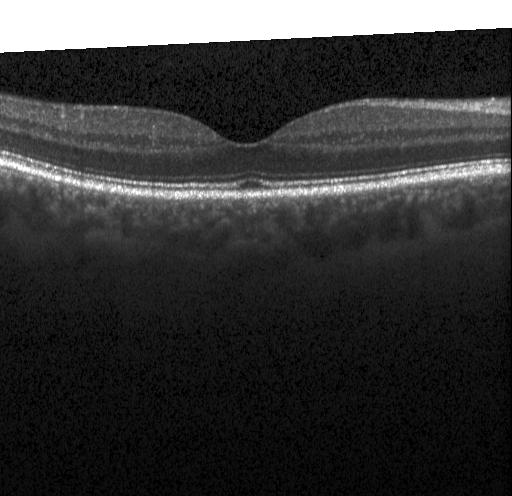

The scan shows neither choroidal neovascularization, diabetic macular edema, nor drusen.